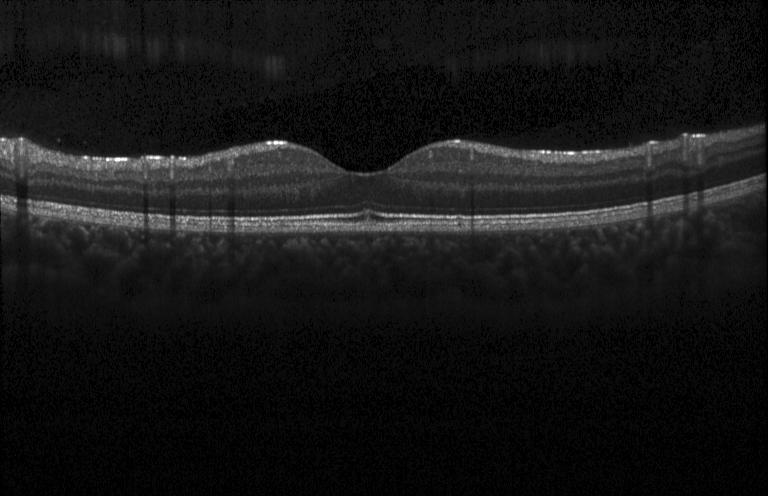 OCT line scan
The scan shows no evidence of choroidal neovascularization, diabetic macular edema, or drusen.